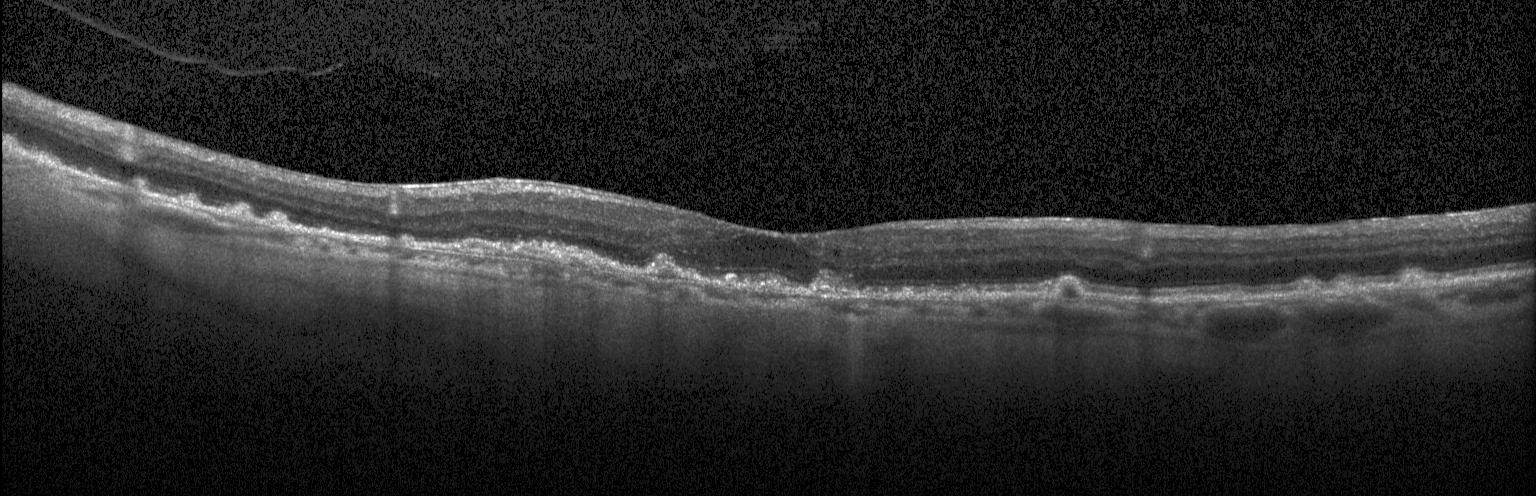

OCT line scan — Assessment: a choroidal neovascular membrane.